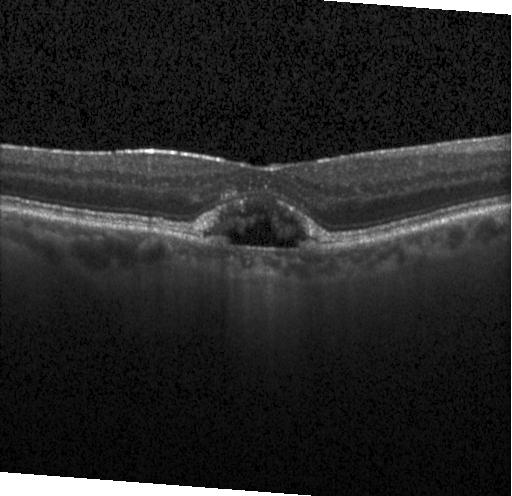 Spectral-domain OCT B-scan: a choroidal neovascular membrane.